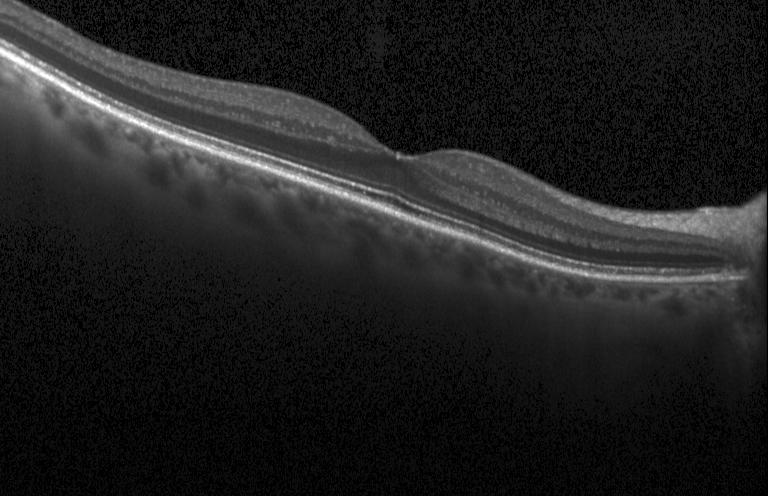
OCT finding: no choroidal neovascularization, diabetic macular edema, or drusen.